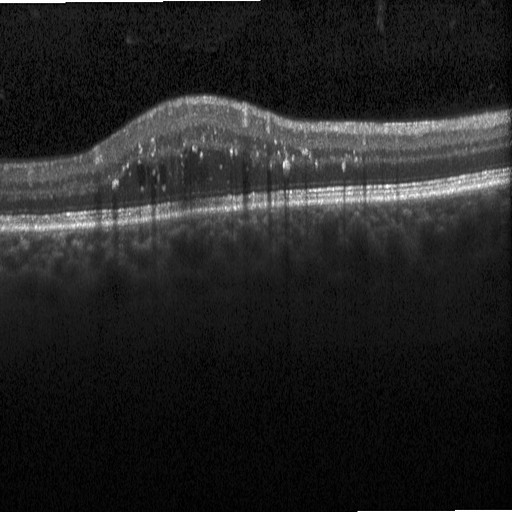
Diagnosis: DME.